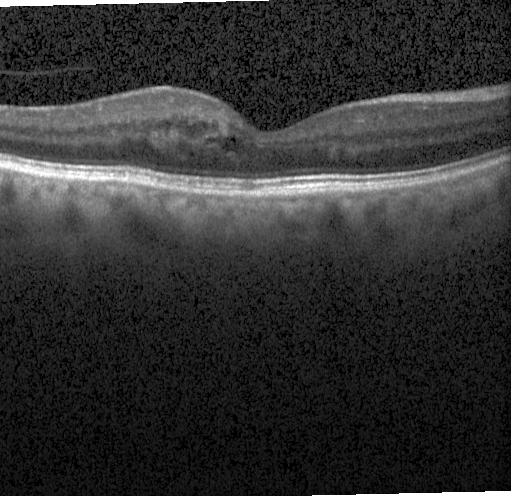
Diagnosis: diabetic macular edema (DME).